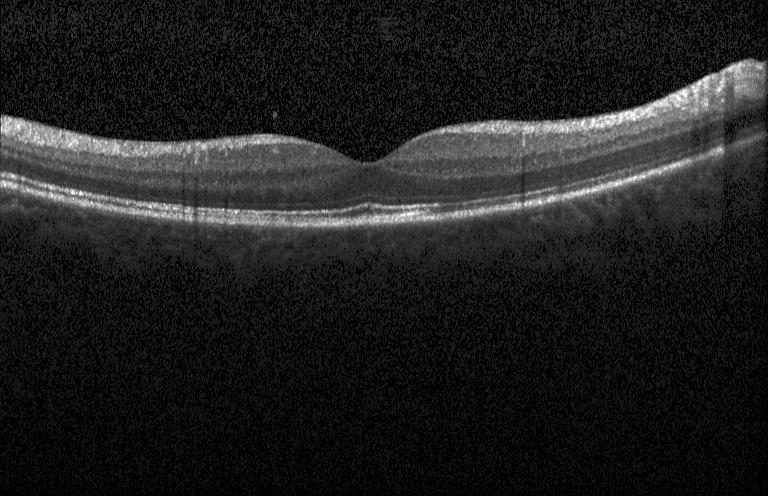 Diagnosis: no evidence of choroidal neovascularization, diabetic macular edema, or drusen.